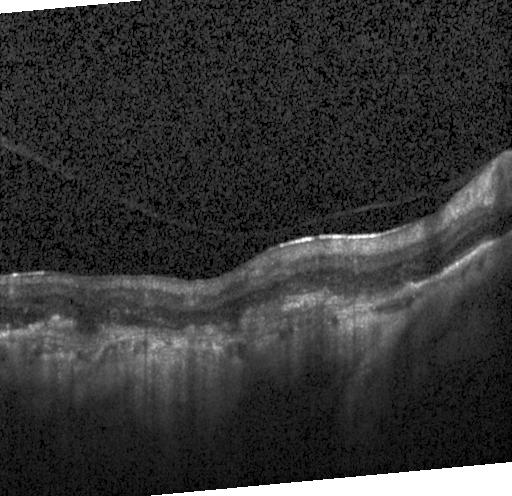 Heidelberg Spectralis OCT system, retinal OCT B-scan — Diagnosis: a choroidal neovascular membrane.